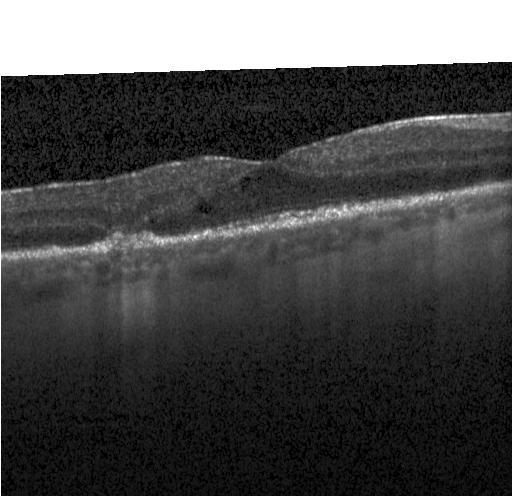

Retinal OCT B-scan; Heidelberg Spectralis OCT system — This B-scan demonstrates a choroidal neovascular membrane.